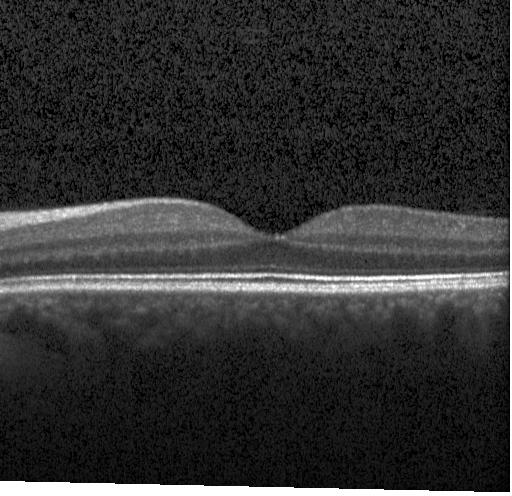 Centered on the fovea; Heidelberg Spectralis OCT system; spectral-domain optical coherence tomography; optical coherence tomography scan
Diagnosis: no evidence of choroidal neovascularization, diabetic macular edema, or drusen.